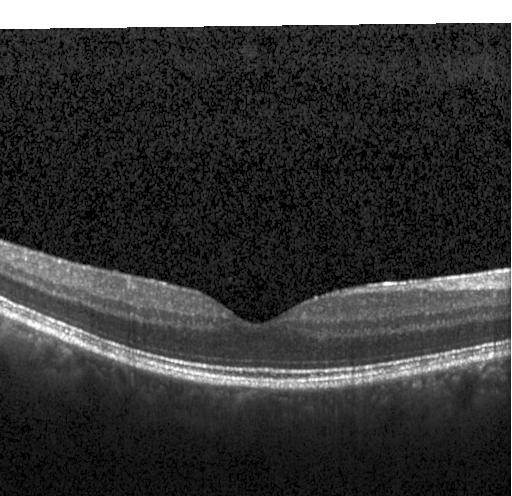
Optical coherence tomography B-scan, through the macula, spectral-domain OCT, instrument: Heidelberg Spectralis
No evidence of choroidal neovascularization, diabetic macular edema, or drusen.